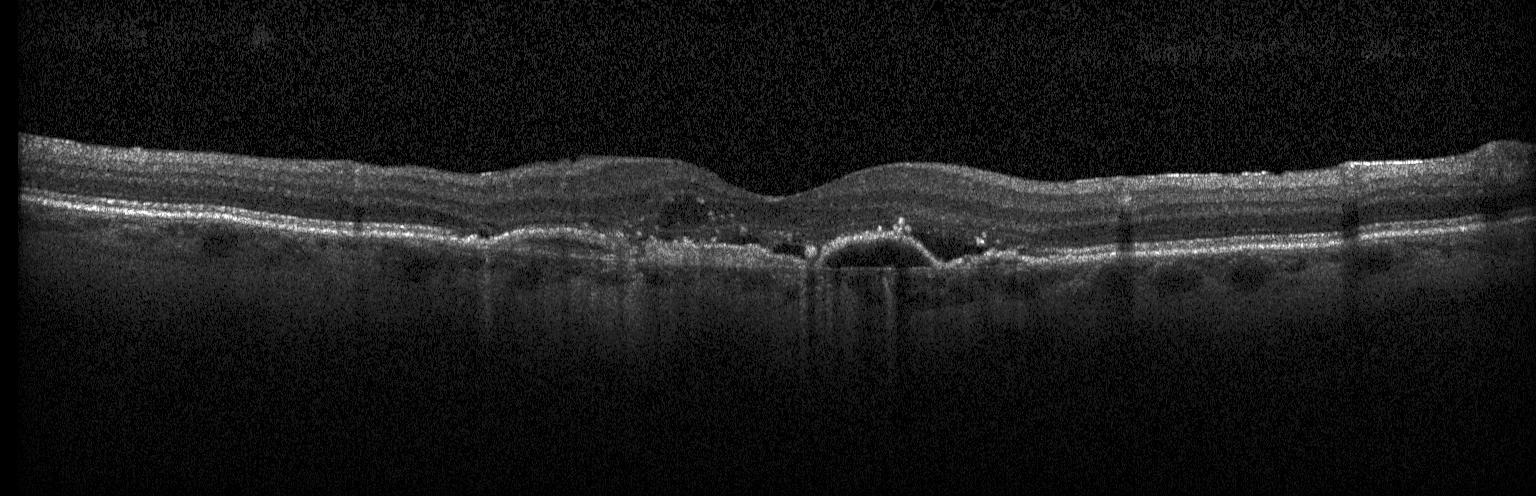

OCT B-scan. Assessment: a choroidal neovascular membrane.